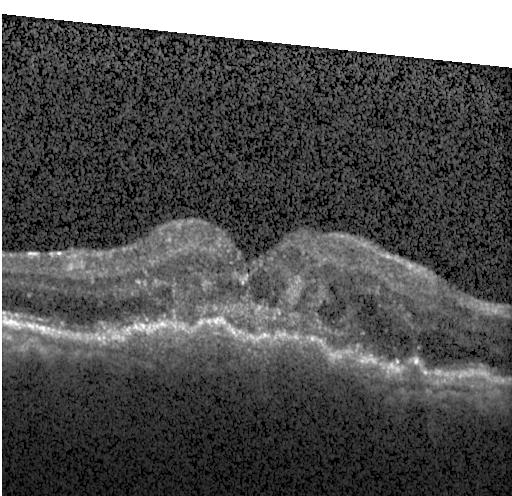

Impression: CNV.